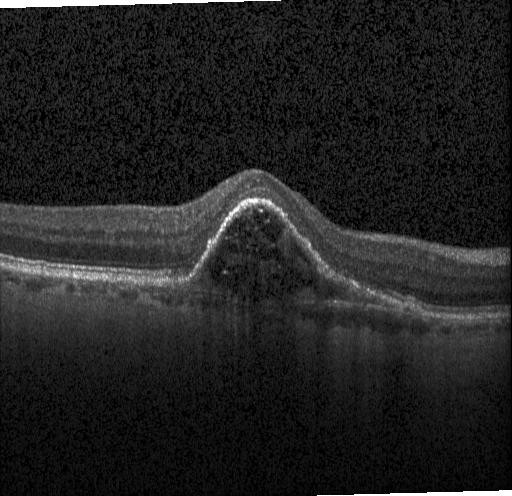

Optical coherence tomography B-scan, fovea-centered, spectral-domain optical coherence tomography — The scan shows choroidal neovascularization (CNV).